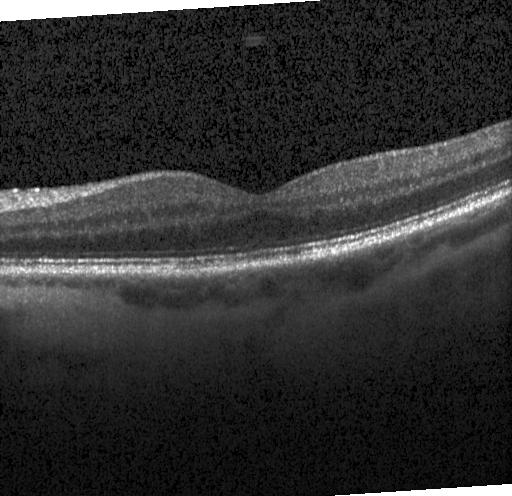
Optical coherence tomography scan
This B-scan demonstrates no evidence of choroidal neovascularization, diabetic macular edema, or drusen.